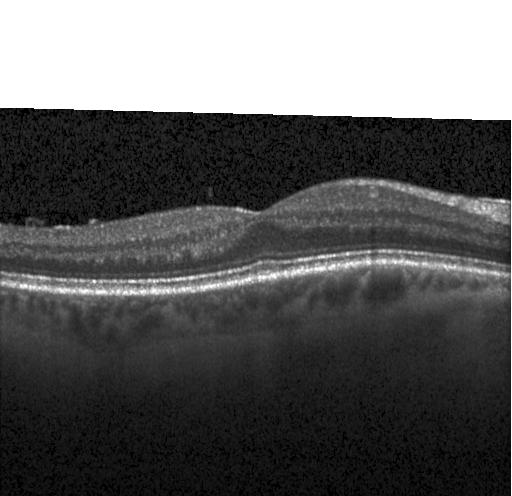 OCT line scan, Heidelberg Spectralis OCT system. Diagnosis: neither choroidal neovascularization, diabetic macular edema, nor drusen.